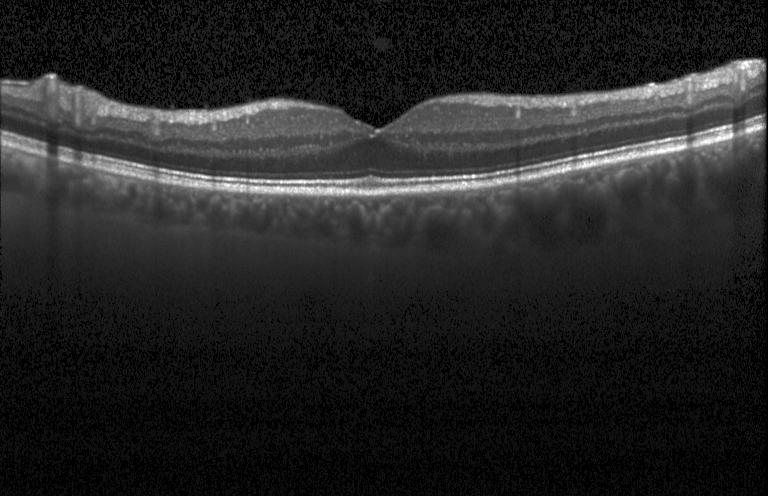 Spectral-domain OCT. Fovea-centered. OCT line scan
Finding: no choroidal neovascularization, diabetic macular edema, or drusen.